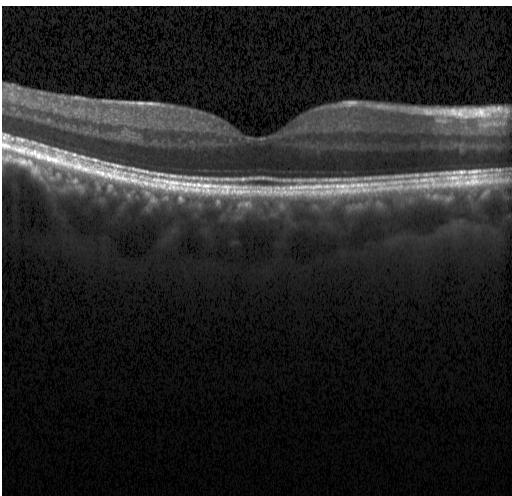

Spectral-domain OCT, OCT B-scan
Neither CNV, DME, nor drusen.